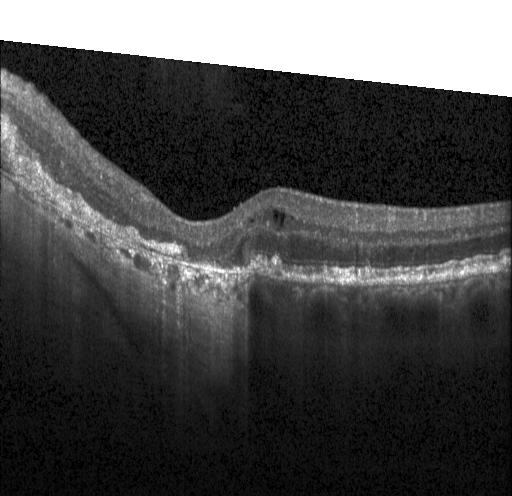 Optical coherence tomography B-scan.
Dx: a choroidal neovascular membrane.